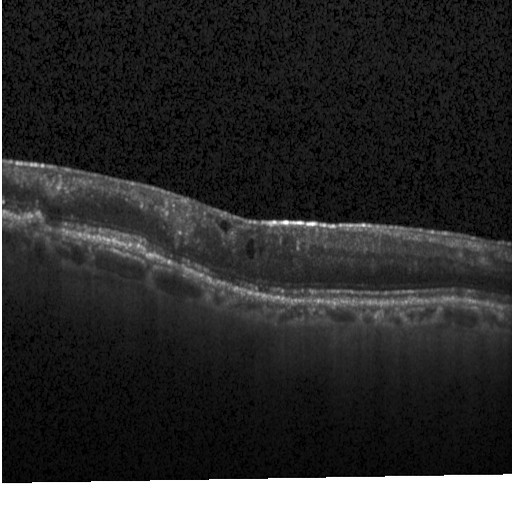
Optical coherence tomography B-scan · instrument: Heidelberg Spectralis — Finding: diabetic macular edema (DME).